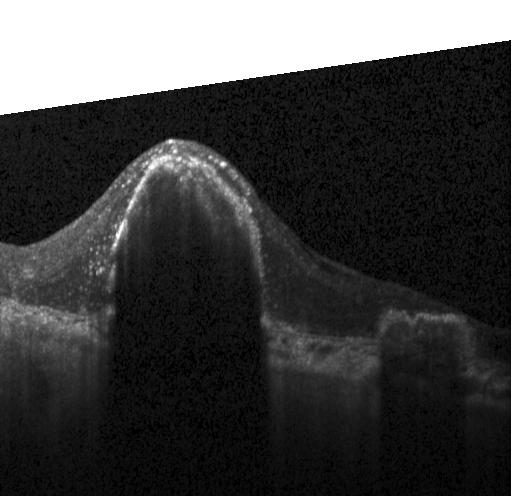 Instrument: Heidelberg Spectralis. Horizontal scan through the fovea. Optical coherence tomography scan. Spectral-domain optical coherence tomography. Diagnosis: choroidal neovascularization.